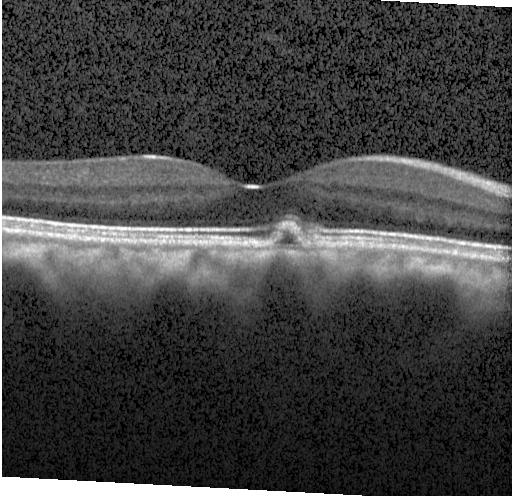

Fovea-centered; SD-OCT; instrument: Heidelberg Spectralis; OCT B-scan
This B-scan demonstrates multiple drusen.